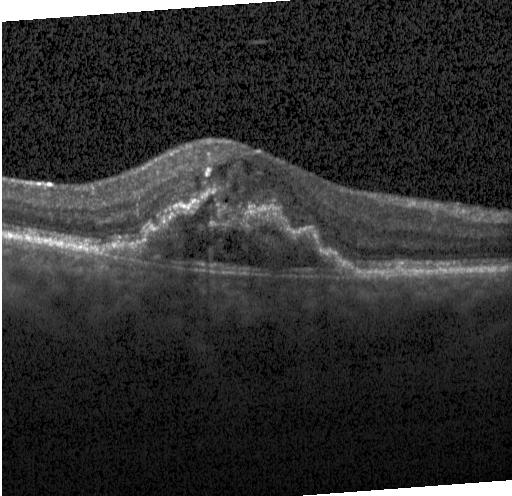
Heidelberg Spectralis, OCT line scan, horizontal scan through the fovea, spectral-domain optical coherence tomography — Impression: CNV.